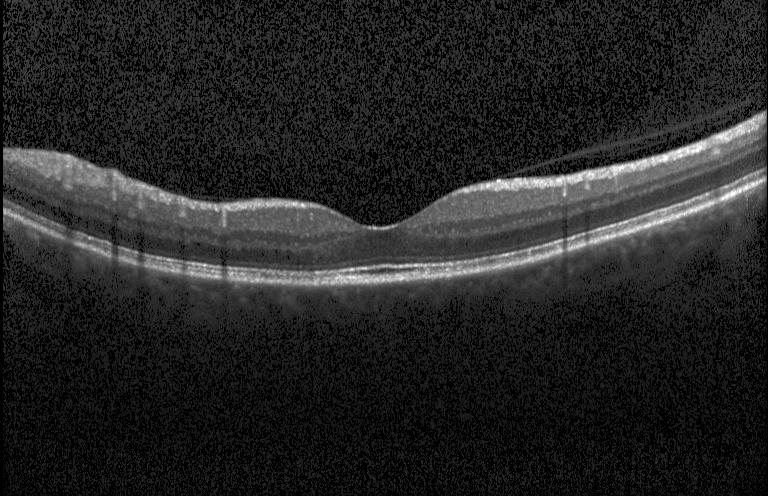 Retinal OCT B-scan; Heidelberg Spectralis OCT system; through the macula. OCT finding: no choroidal neovascularization, diabetic macular edema, or drusen.